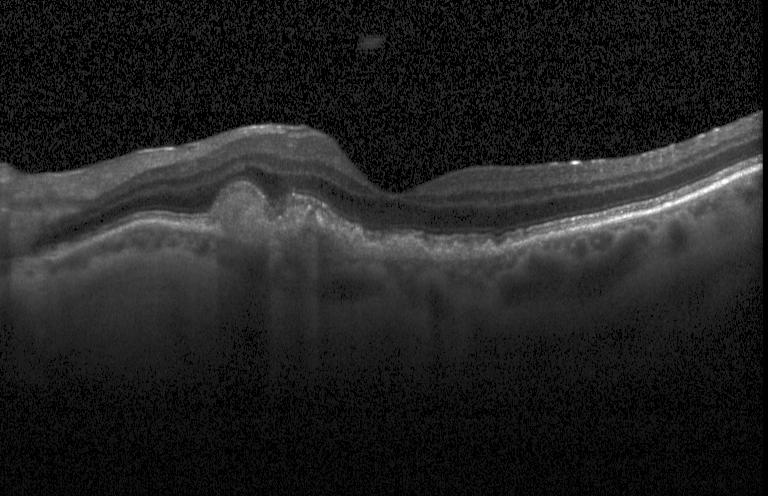

Spectral-domain OCT. Retinal OCT B-scan — Dx: CNV.